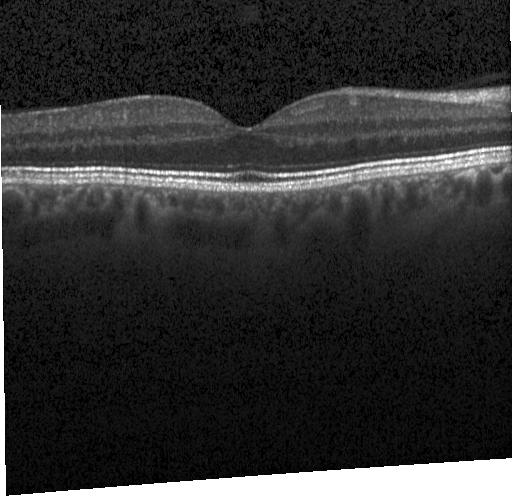 Impression: neither choroidal neovascularization, diabetic macular edema, nor drusen.